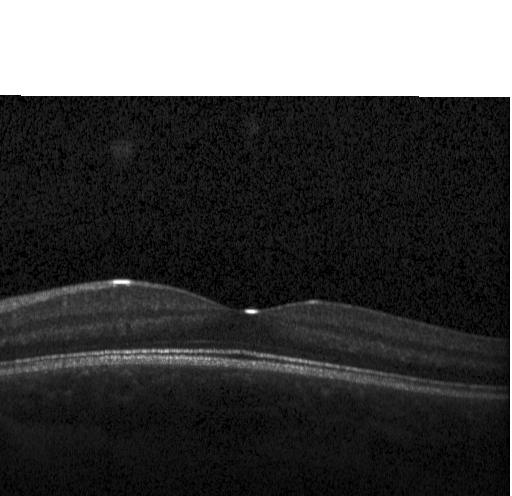 Retinal OCT B-scan
Assessment: no evidence of choroidal neovascularization, diabetic macular edema, or drusen.